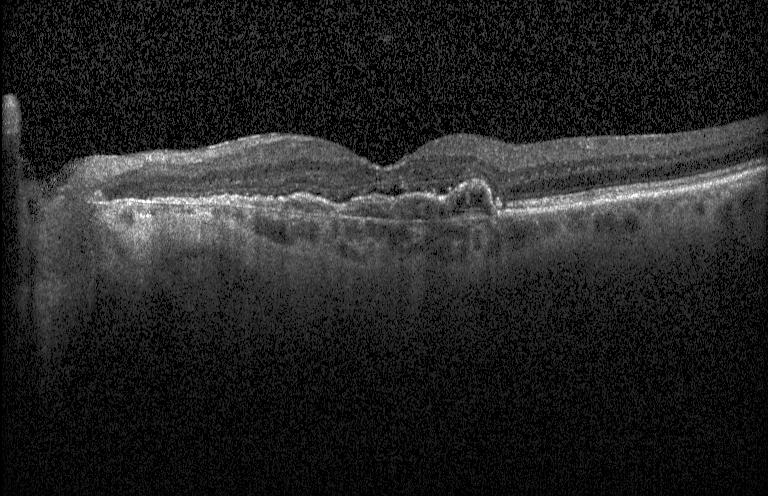

OCT B-scan, SD-OCT — Macular OCT: a choroidal neovascular membrane.